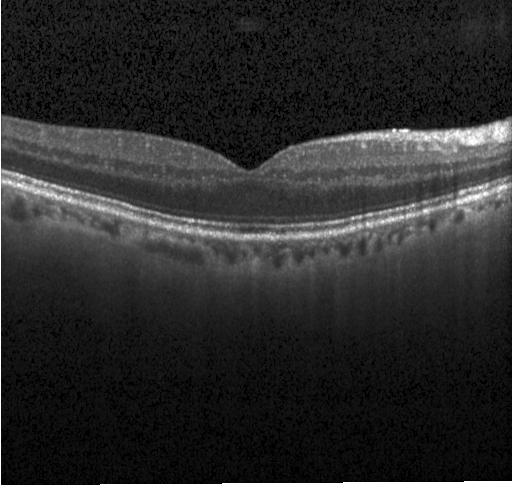 OCT line scan. Instrument: Heidelberg Spectralis. OCT finding: no evidence of choroidal neovascularization, diabetic macular edema, or drusen.